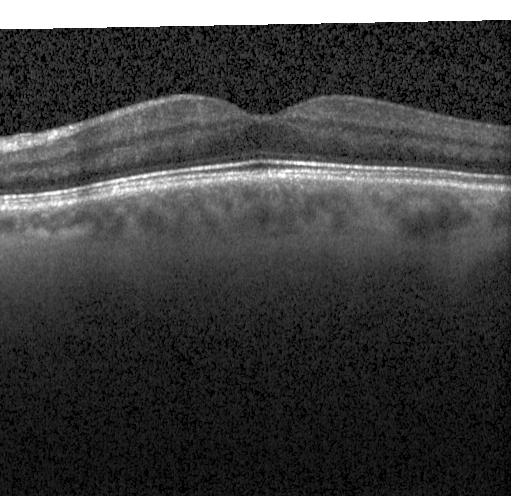 Optical coherence tomography B-scan
Finding: neither choroidal neovascularization, diabetic macular edema, nor drusen.